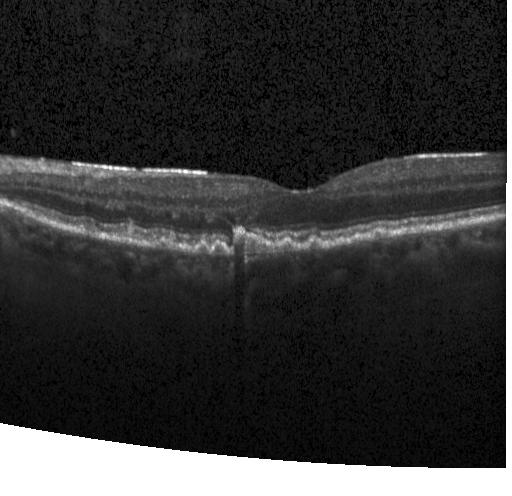
Heidelberg Spectralis OCT system, OCT line scan, fovea-centered, SD-OCT. The scan shows a choroidal neovascular membrane.